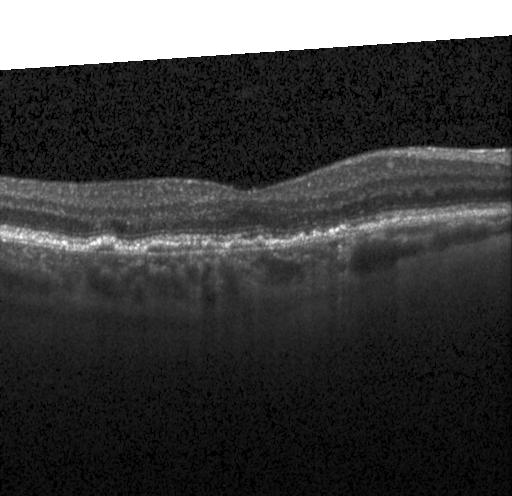 Spectral-domain OCT, centered on the fovea, retinal OCT cross-section. This B-scan demonstrates choroidal neovascularization (CNV).